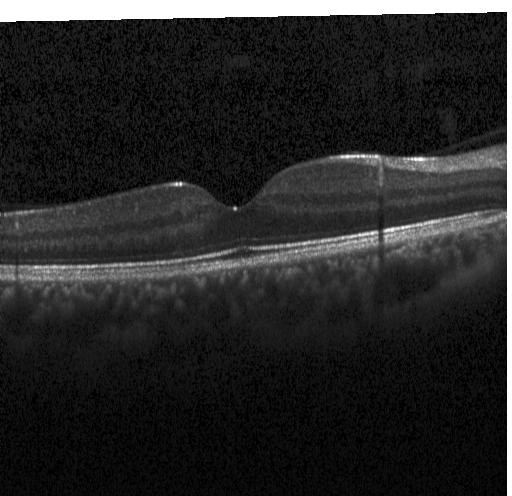
Heidelberg Spectralis OCT system. OCT line scan. Macular scan. Spectral-domain OCT — Finding: no evidence of choroidal neovascularization, diabetic macular edema, or drusen.